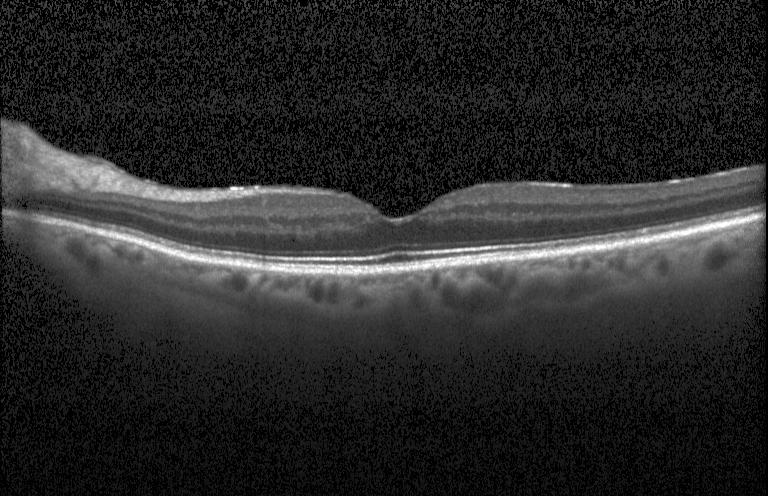

Diagnosis: neither choroidal neovascularization, diabetic macular edema, nor drusen.